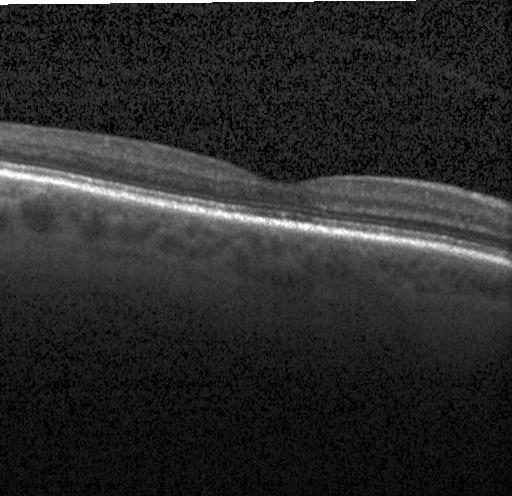 SD-OCT, retinal OCT B-scan
Diagnosis: no CNV, no DME, and no drusen.